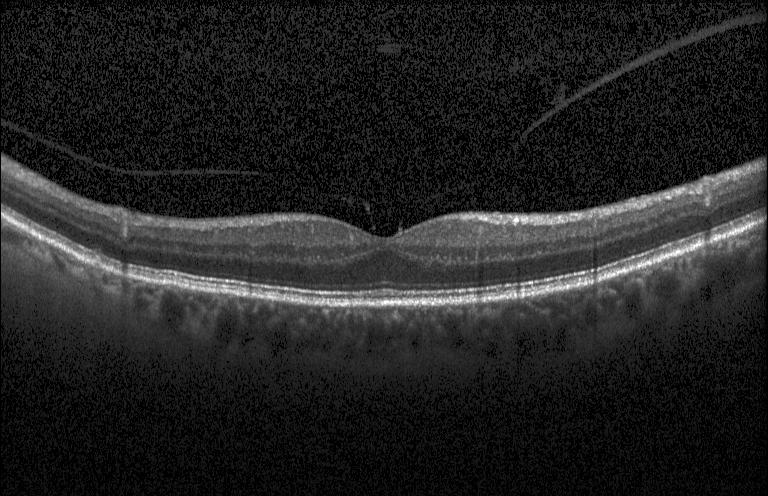

Heidelberg Spectralis, retinal OCT cross-section, through the macula, SD-OCT
Finding: no choroidal neovascularization, diabetic macular edema, or drusen.